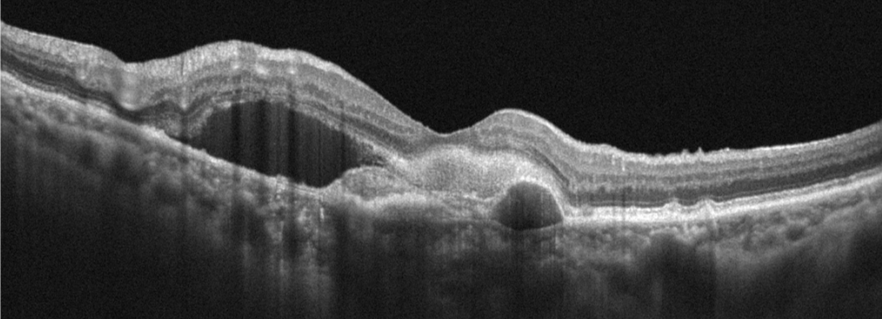

Assessment: AMD.